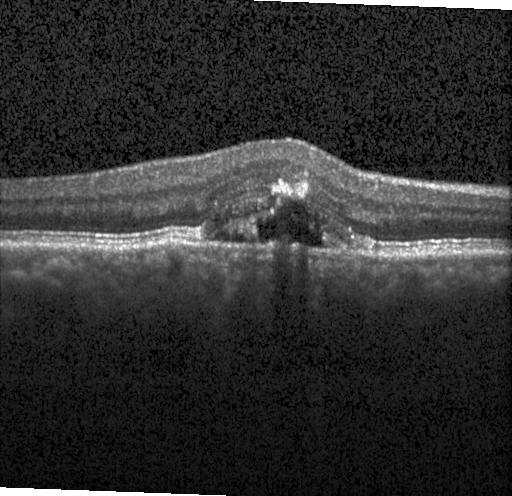
OCT B-scan. Impression: a choroidal neovascular membrane.